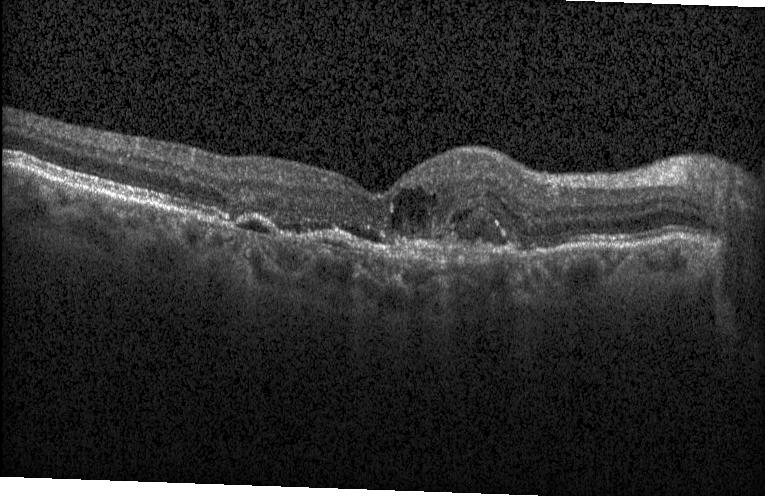
The scan shows choroidal neovascularization (CNV).